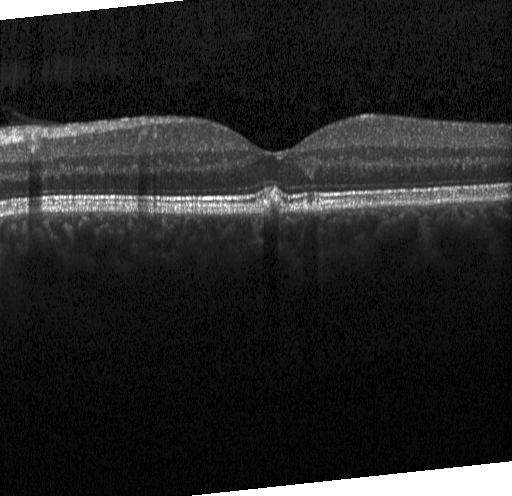 OCT finding: sub-RPE drusenoid deposits.